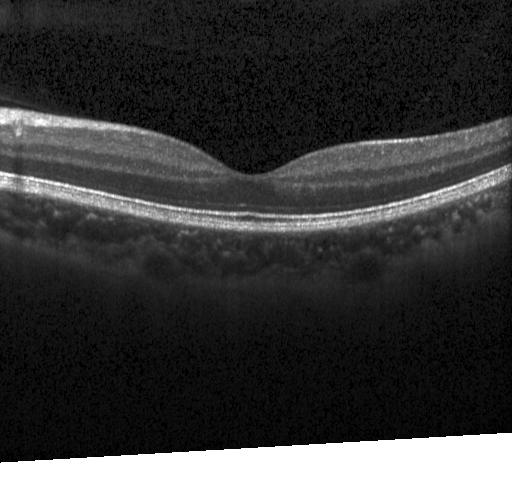
Finding: no CNV, DME, or drusen.